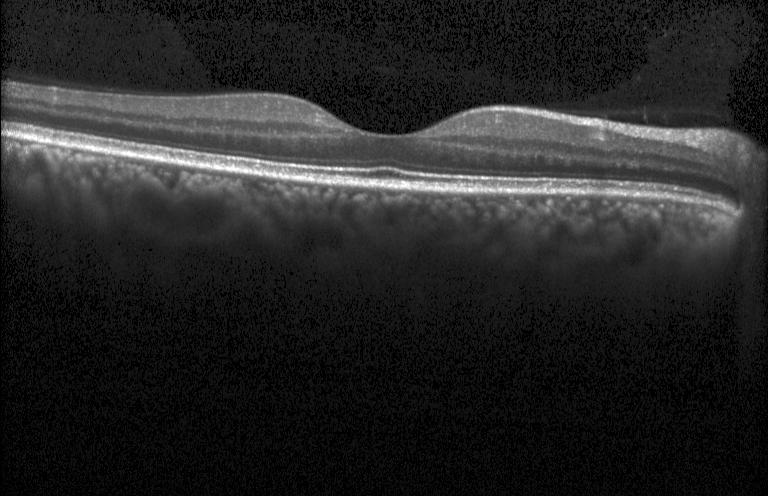
Macular OCT: no CNV, DME, or drusen.